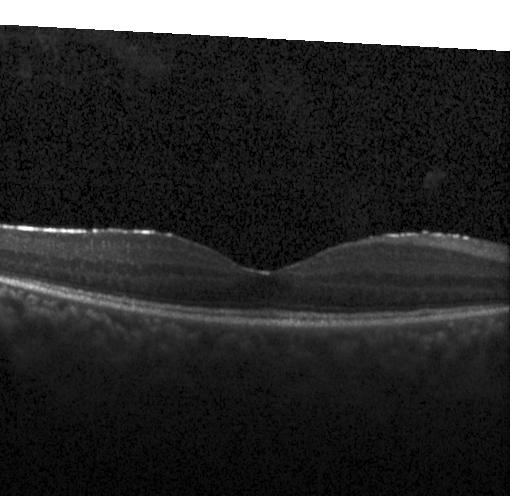

Finding: no evidence of choroidal neovascularization, diabetic macular edema, or drusen.